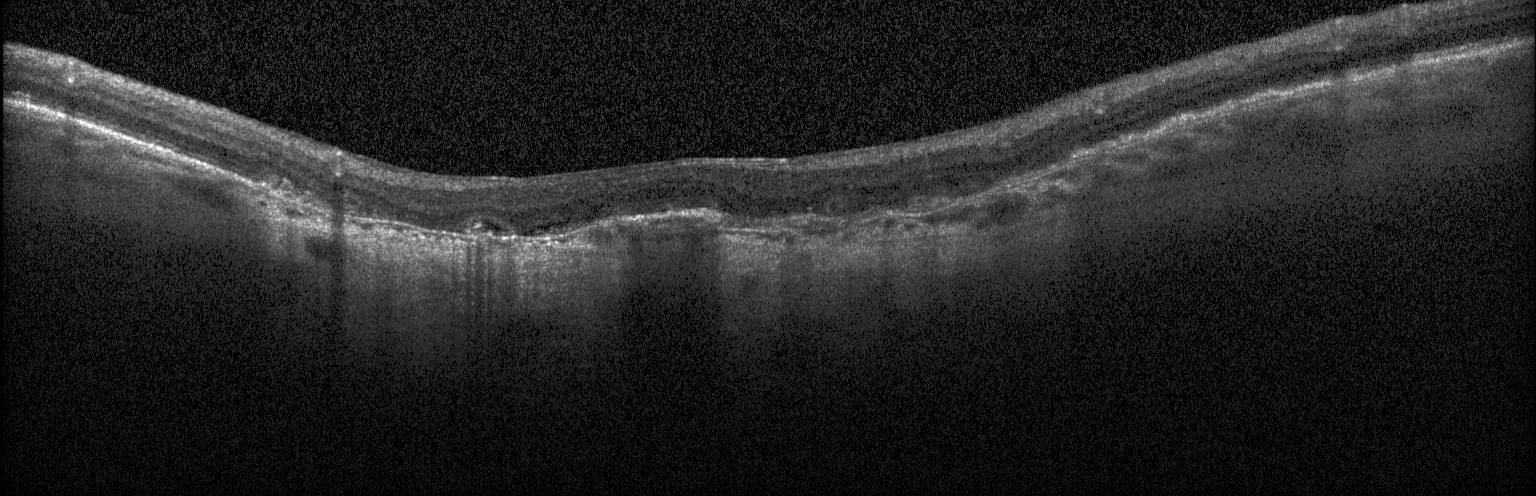

Optical coherence tomography B-scan. This B-scan demonstrates choroidal neovascularization (CNV).